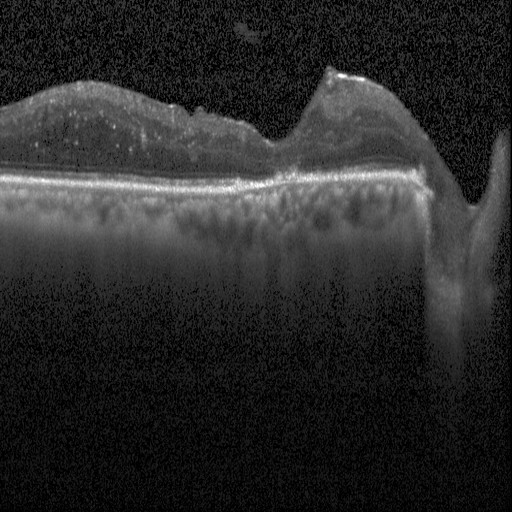
OCT line scan
Assessment: DME.